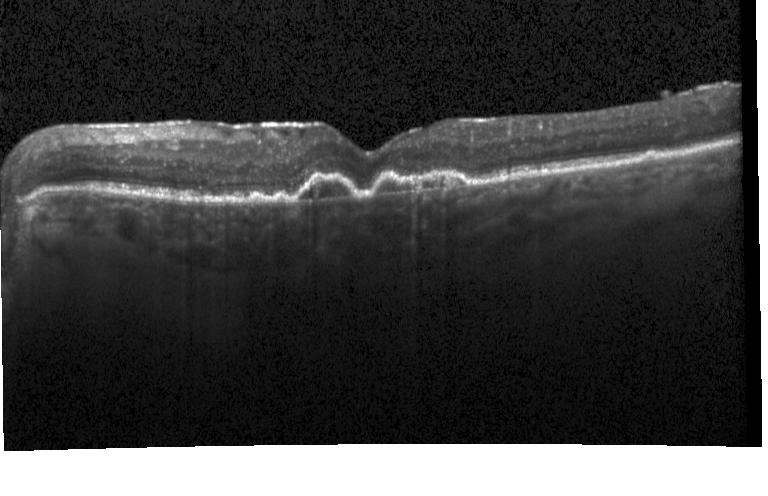
Impression: choroidal neovascularization.